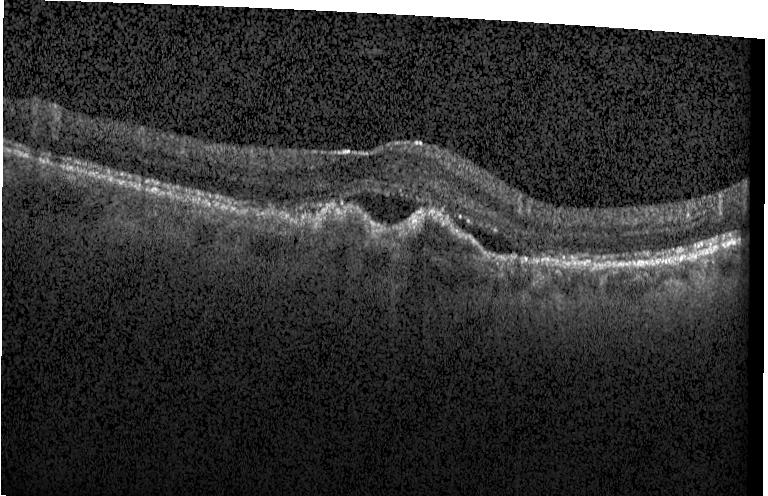 Diagnosis: choroidal neovascularization (CNV).